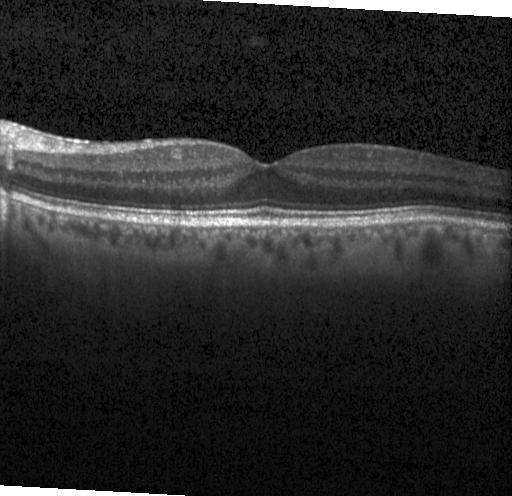

Macular scan. OCT B-scan. Spectral-domain optical coherence tomography. This B-scan demonstrates no choroidal neovascularization, diabetic macular edema, or drusen.